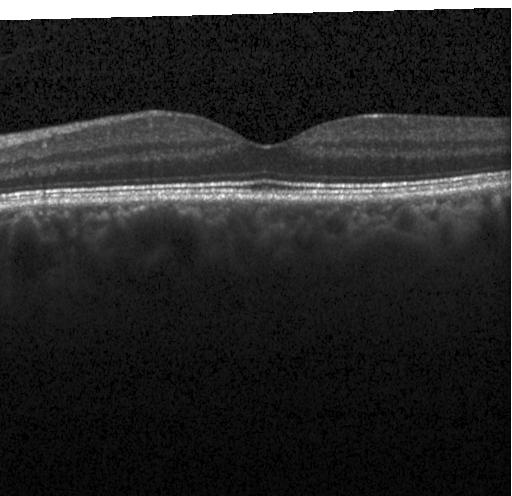

Optical coherence tomography B-scan · spectral-domain OCT. Dx: neither choroidal neovascularization, diabetic macular edema, nor drusen.